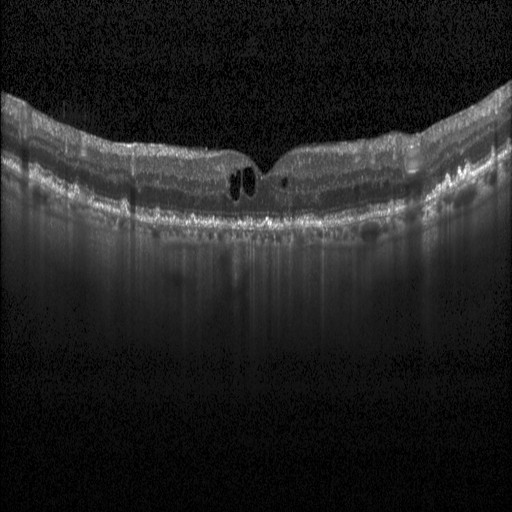

Spectral-domain OCT; instrument: Heidelberg Spectralis; OCT B-scan — Diagnosis: diabetic macular edema (DME).